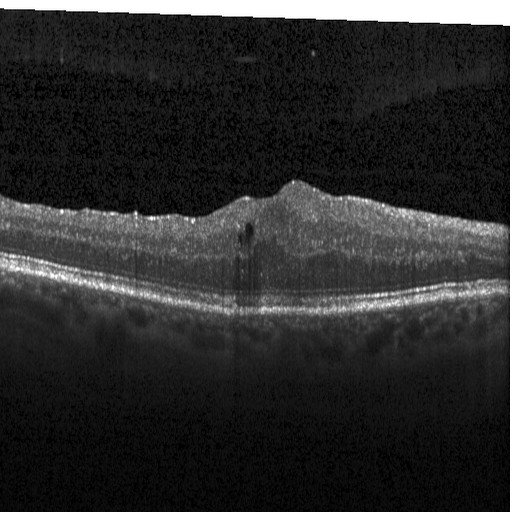

Retinal OCT cross-section; through the macula; Heidelberg Spectralis OCT system; spectral-domain OCT — Diagnosis: DME.